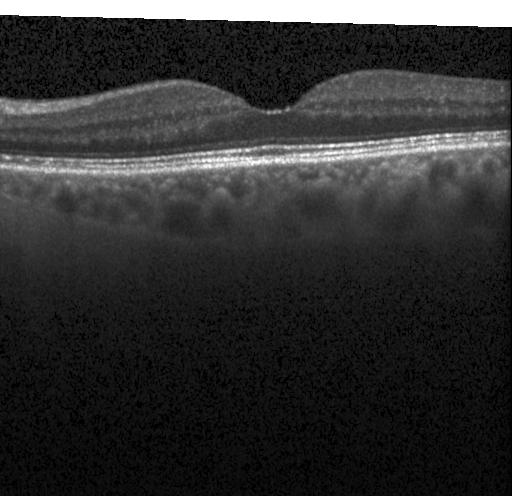 Finding: no choroidal neovascularization, no diabetic macular edema, and no drusen.